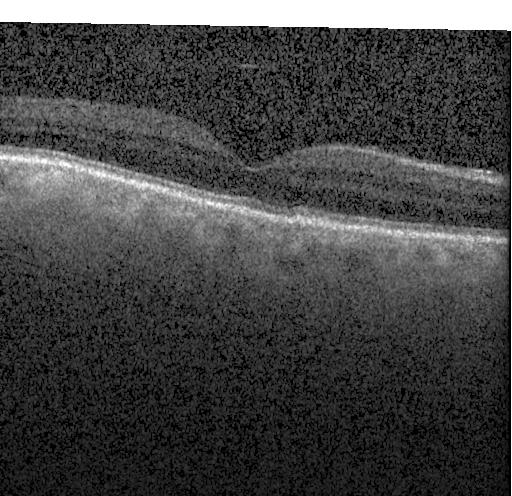 Optical coherence tomography B-scan. Assessment: no evidence of choroidal neovascularization, diabetic macular edema, or drusen.